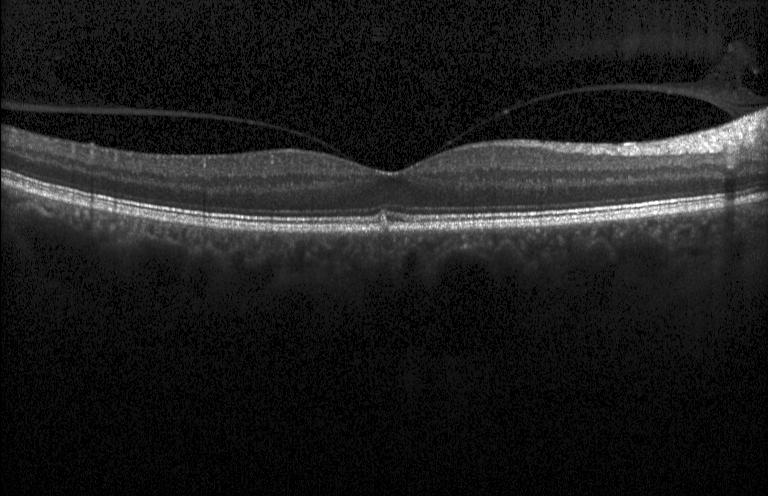

The scan shows multiple drusen.